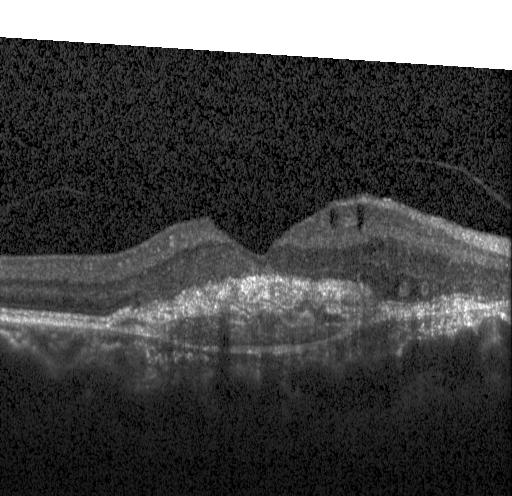

Spectral-domain optical coherence tomography · OCT B-scan · fovea-centered — Impression: a choroidal neovascular membrane.